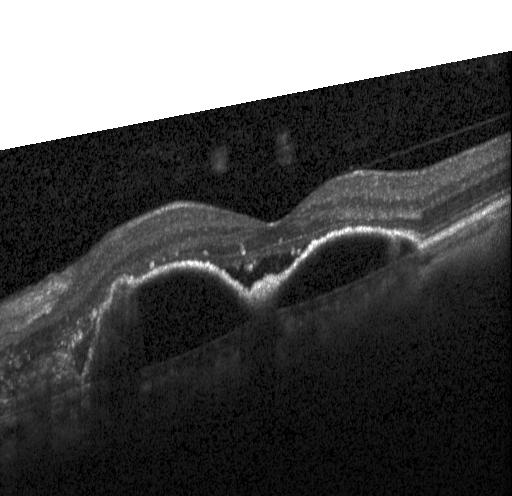
Finding: choroidal neovascularization (CNV).